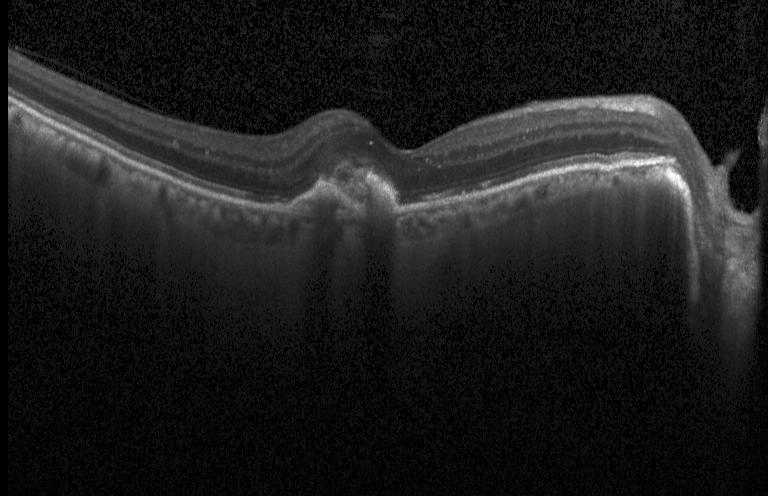

Spectral-domain OCT B-scan: choroidal neovascularization (CNV).